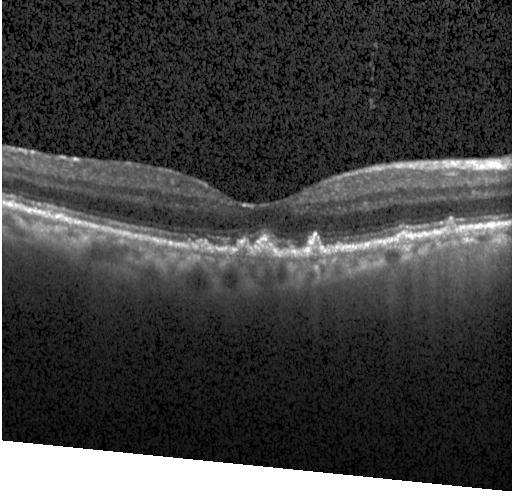

Optical coherence tomography B-scan
This B-scan demonstrates drusen.